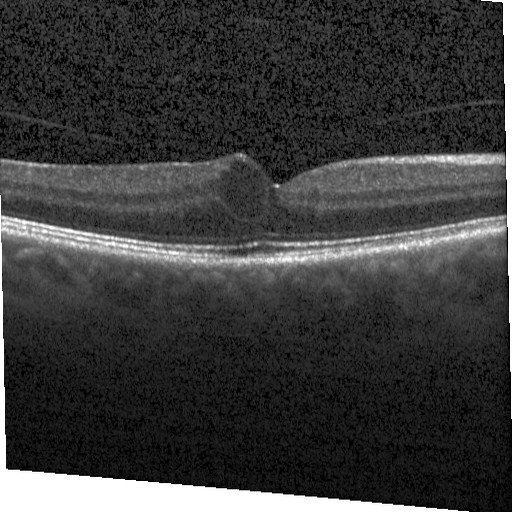
Spectral-domain OCT · retinal OCT cross-section · instrument: Heidelberg Spectralis.
Impression: diabetic macular edema (DME).